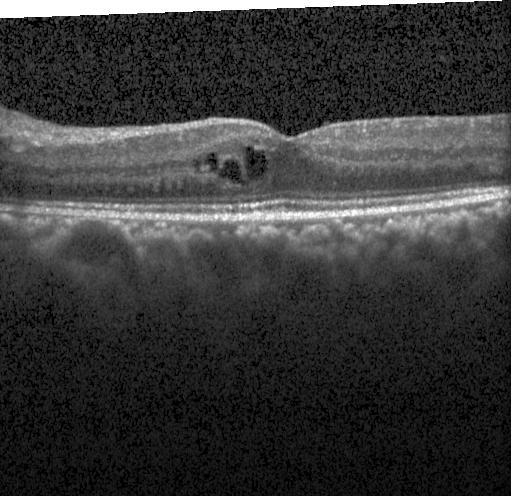

Finding: diabetic macular edema (DME).